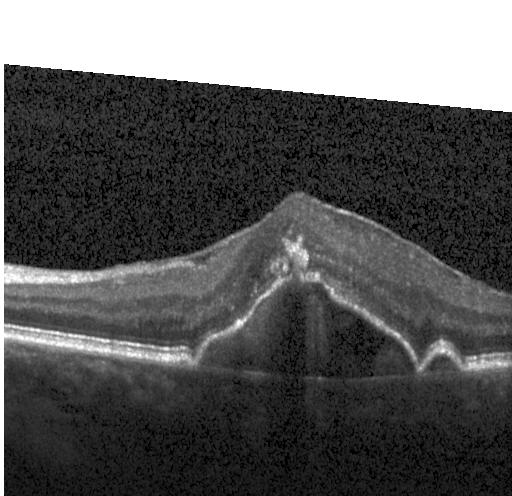
Finding: a choroidal neovascular membrane.